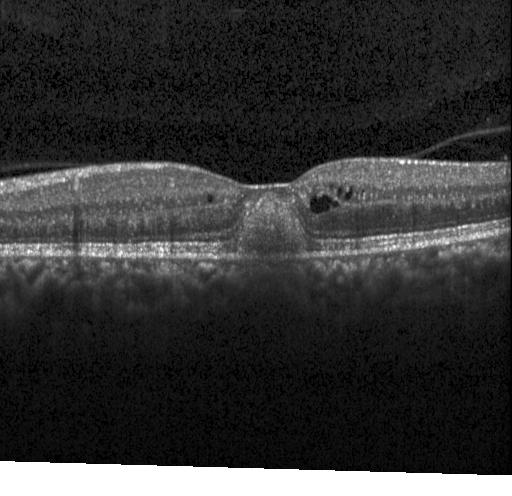
Impression: CNV.